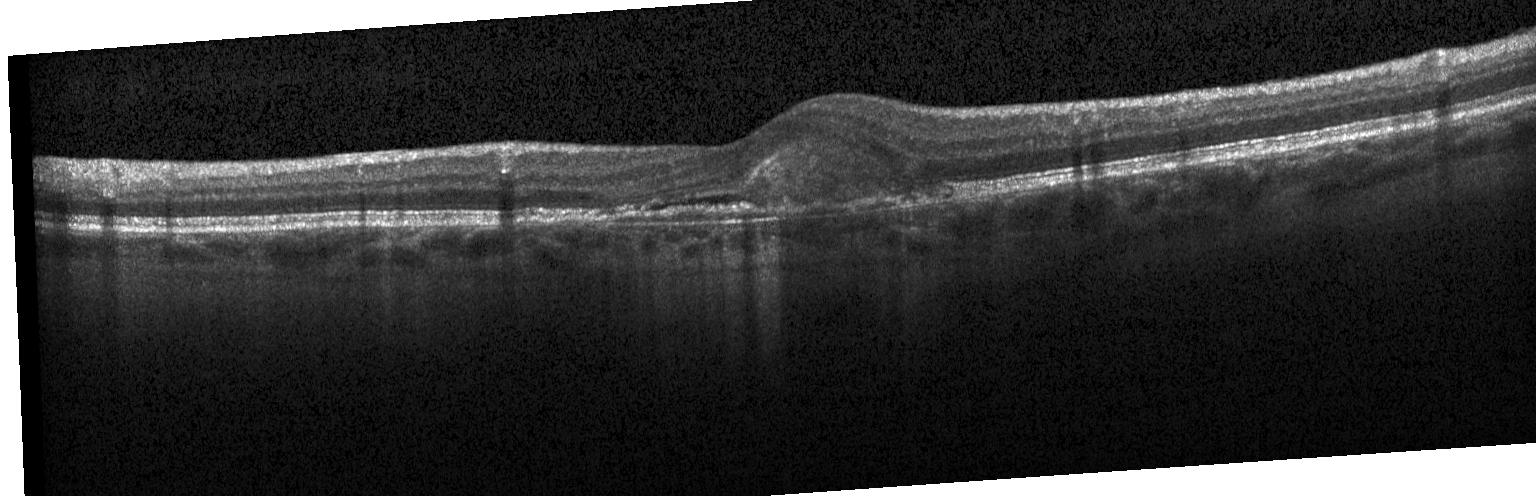 Impression: CNV.